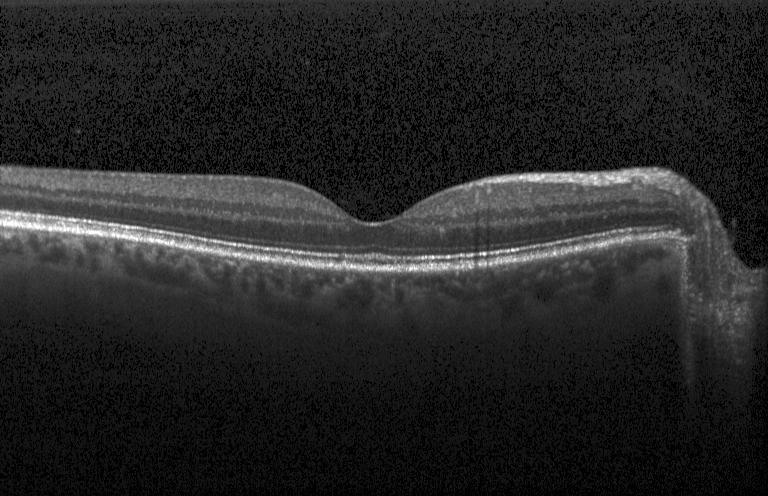 OCT B-scan showing no evidence of choroidal neovascularization, diabetic macular edema, or drusen.